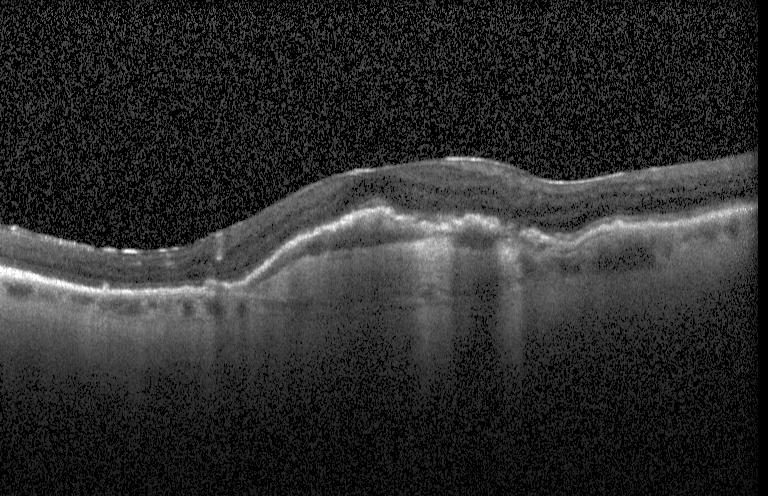 Finding: a choroidal neovascular membrane.